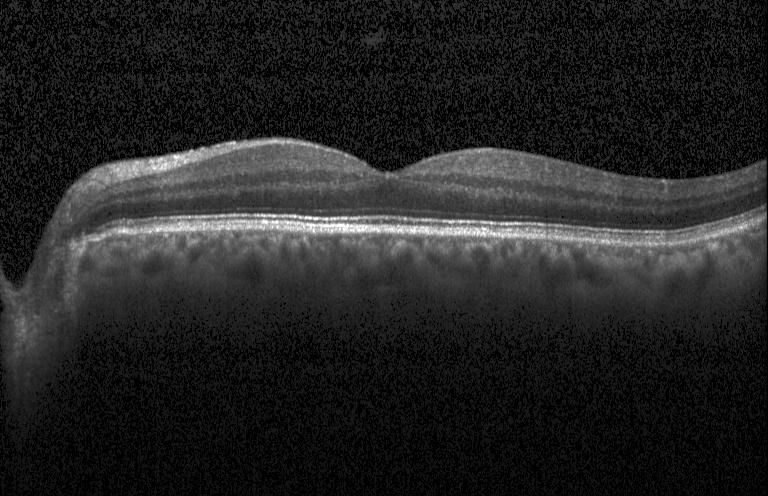
Heidelberg Spectralis. OCT B-scan. This B-scan demonstrates no choroidal neovascularization, no diabetic macular edema, and no drusen.